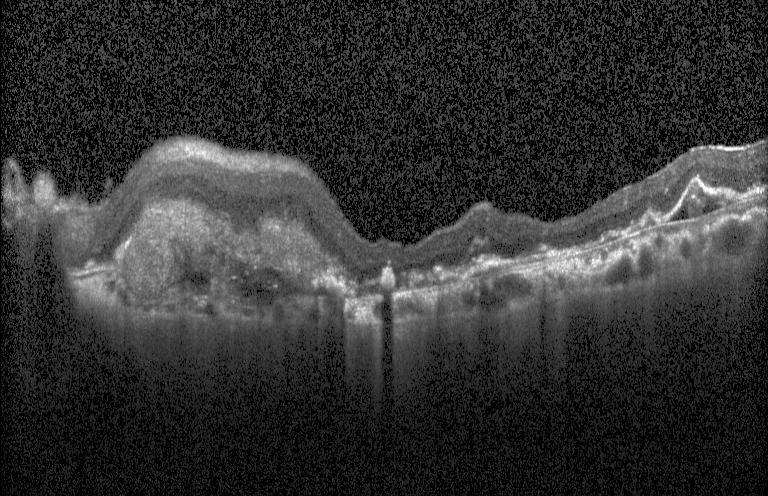 Diagnosis: choroidal neovascularization.